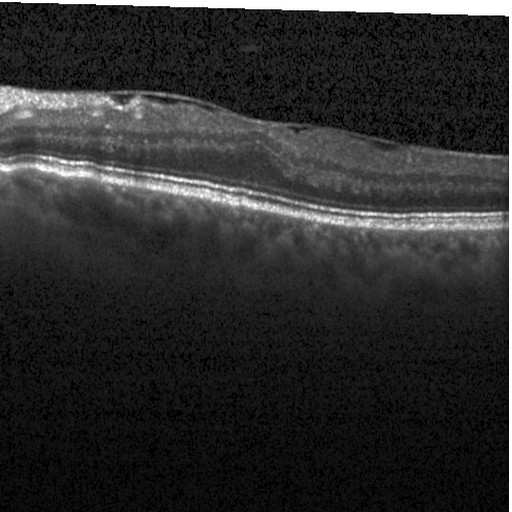 Optical coherence tomography B-scan, SD-OCT, centered on the fovea.
The scan shows DME.